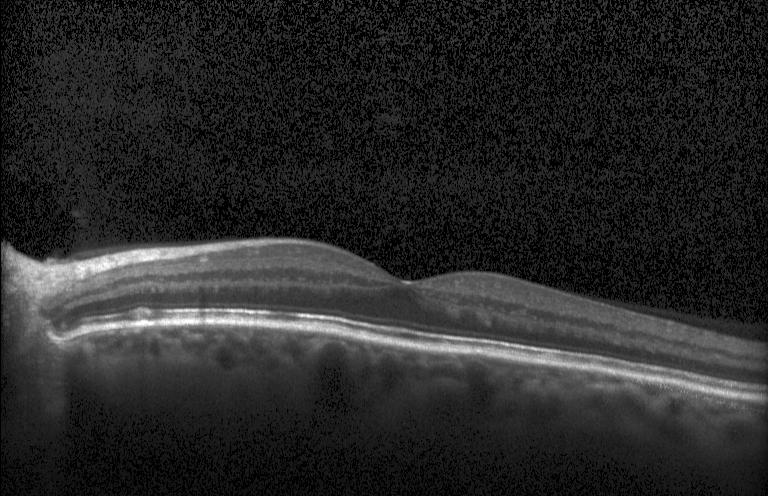

Spectral-domain OCT. Heidelberg Spectralis OCT system. Retinal OCT cross-section. Horizontal scan through the fovea — Finding: no evidence of CNV, DME, or drusen.